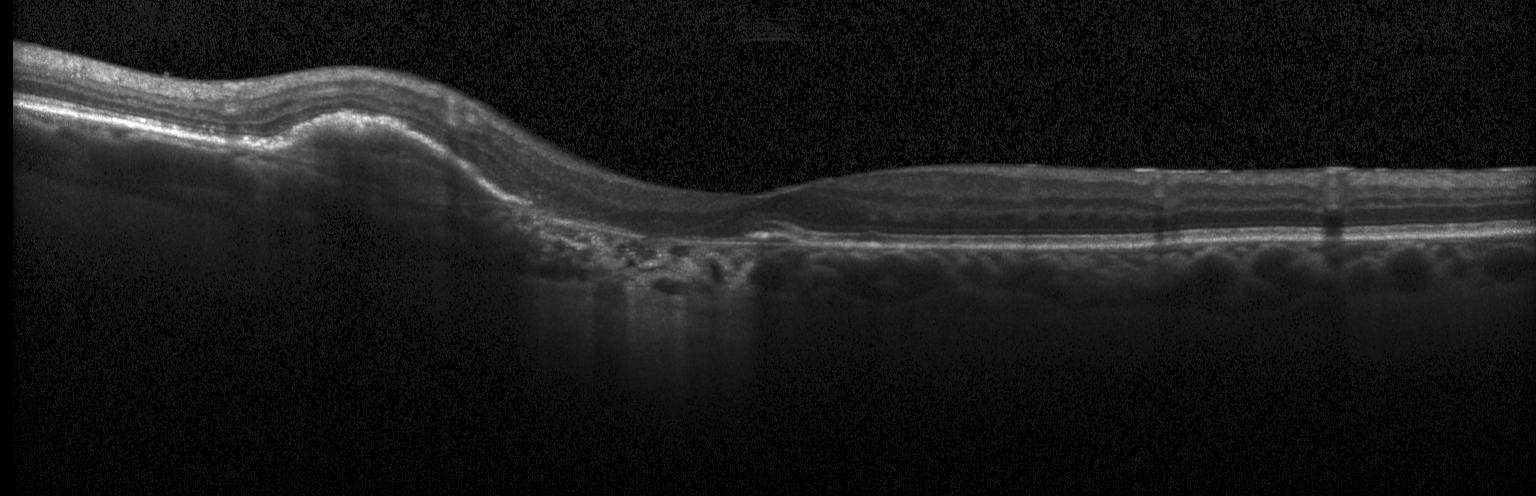 Heidelberg Spectralis OCT system, OCT line scan, centered on the fovea. Finding: a choroidal neovascular membrane.